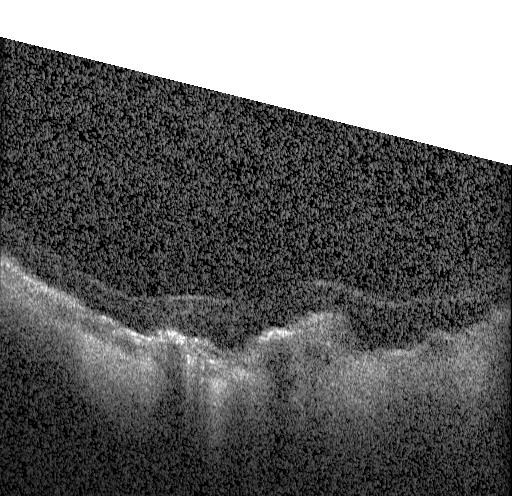 Instrument: Heidelberg Spectralis. Centered on the fovea. Optical coherence tomography B-scan. A choroidal neovascular membrane.